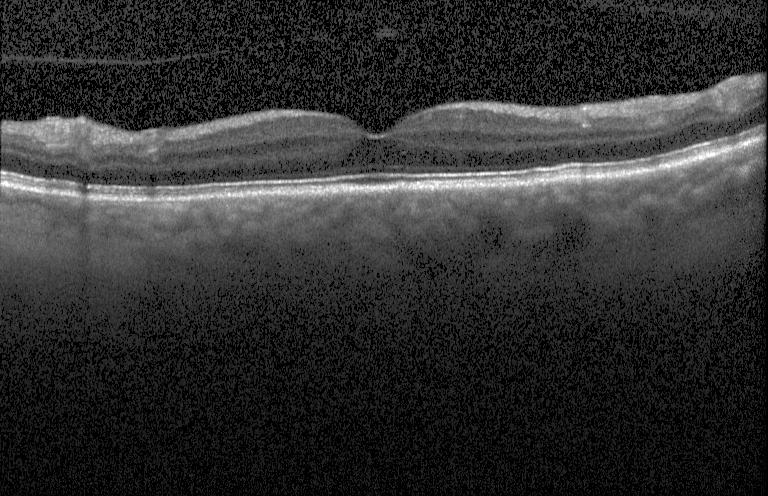

Optical coherence tomography B-scan. Heidelberg Spectralis OCT system. Assessment: neither choroidal neovascularization, diabetic macular edema, nor drusen.